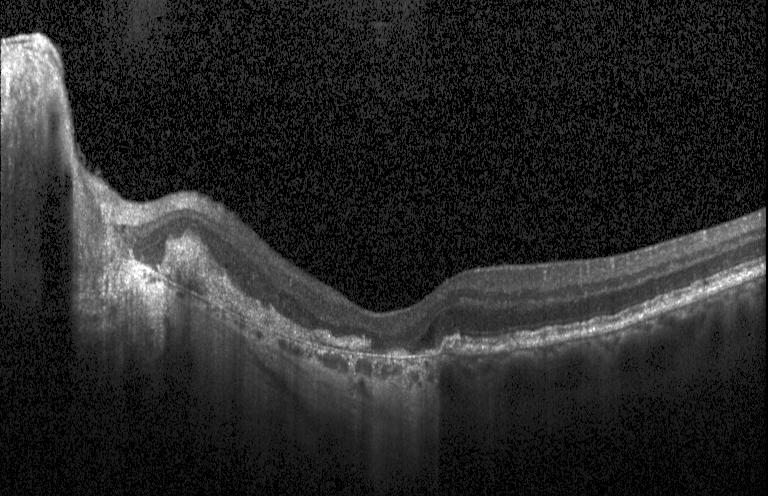

Impression: CNV.